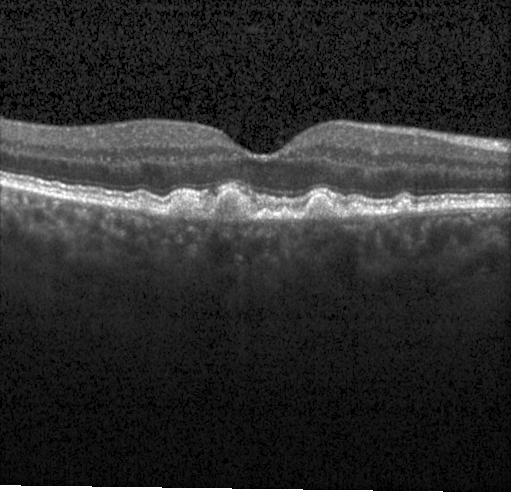
Heidelberg Spectralis OCT system · SD-OCT · centered on the fovea · retinal OCT cross-section.
Assessment: sub-RPE drusenoid deposits.